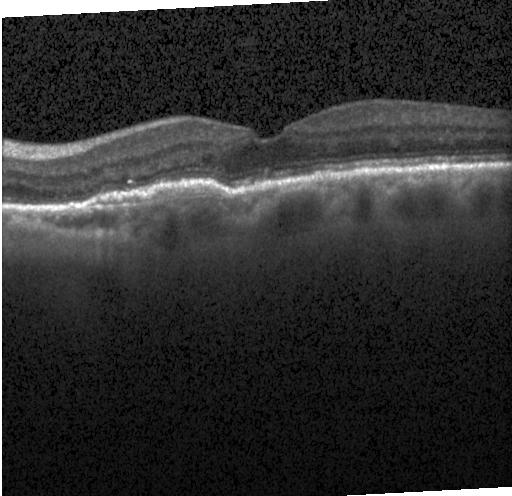 Retinal OCT cross-section showing CNV.